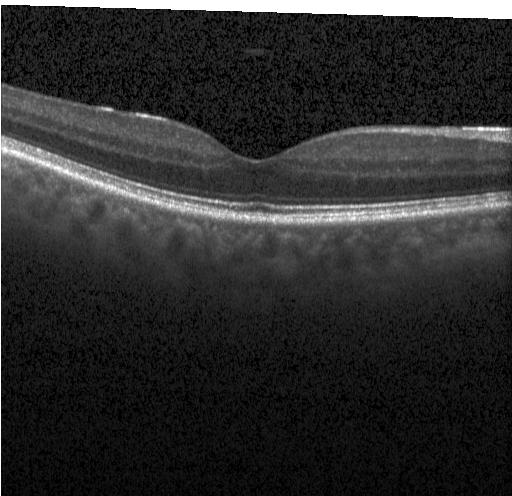

Optical coherence tomography B-scan — No evidence of choroidal neovascularization, diabetic macular edema, or drusen.